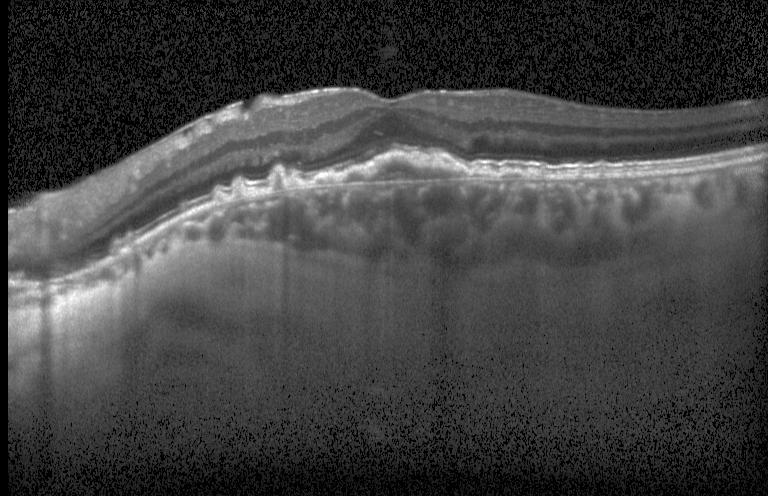
Heidelberg Spectralis OCT system · spectral-domain optical coherence tomography · retinal OCT cross-section. Impression: choroidal neovascularization (CNV).